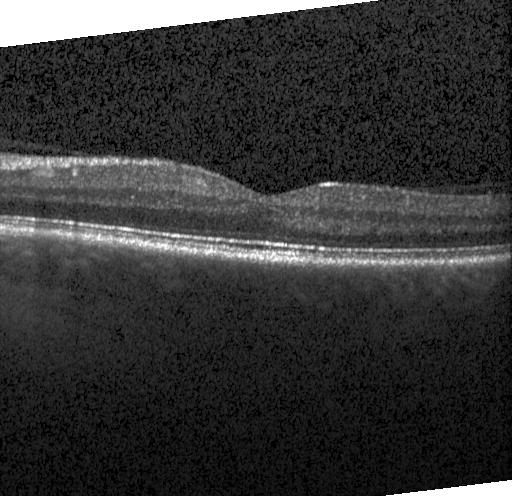
Impression: neither choroidal neovascularization, diabetic macular edema, nor drusen.